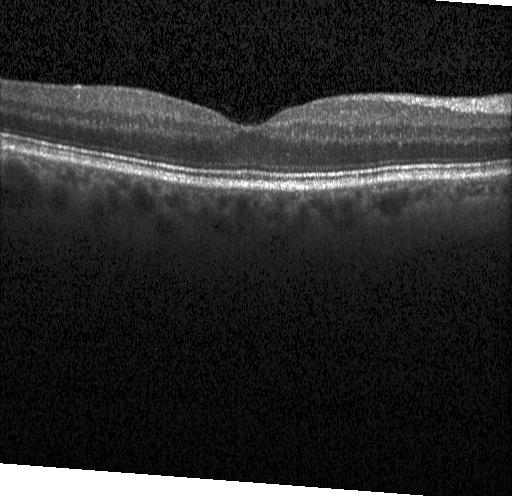

Heidelberg Spectralis · fovea-centered · retinal OCT B-scan — OCT finding: no evidence of choroidal neovascularization, diabetic macular edema, or drusen.